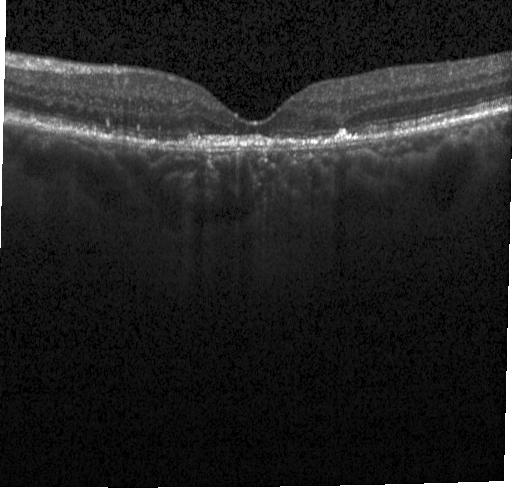 Optical coherence tomography B-scan, spectral-domain OCT.
Impression: choroidal neovascularization.